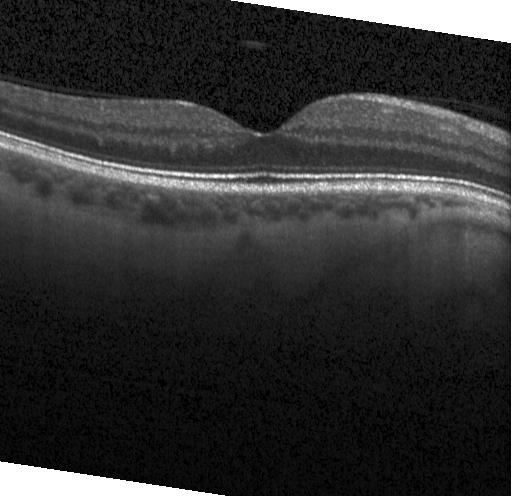

Horizontal scan through the fovea. Heidelberg Spectralis. OCT B-scan.
No evidence of choroidal neovascularization, diabetic macular edema, or drusen.